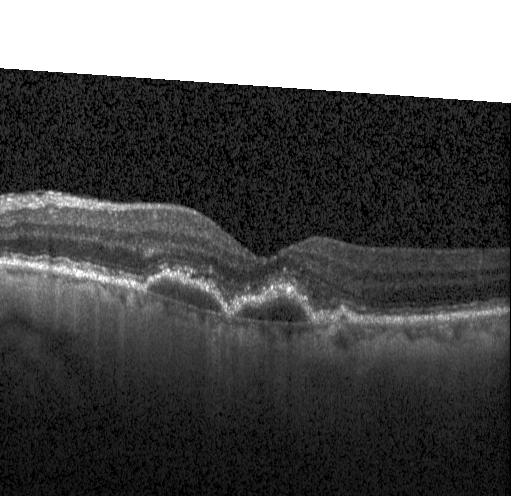
Spectral-domain OCT B-scan: choroidal neovascularization.